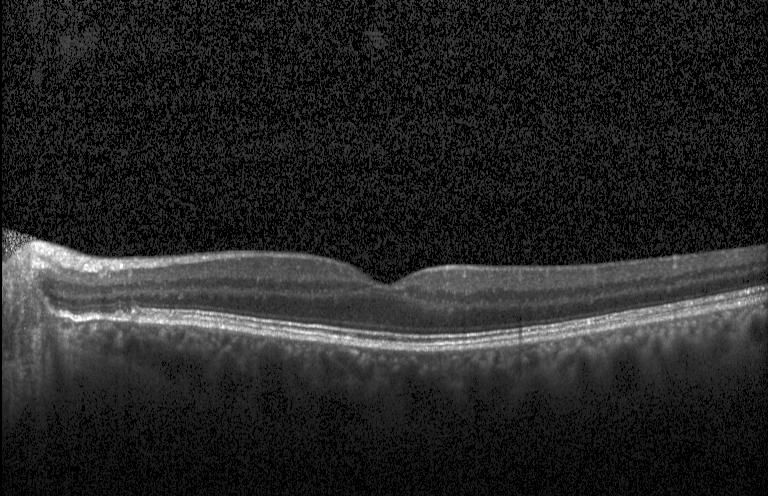

The scan shows no evidence of choroidal neovascularization, diabetic macular edema, or drusen.